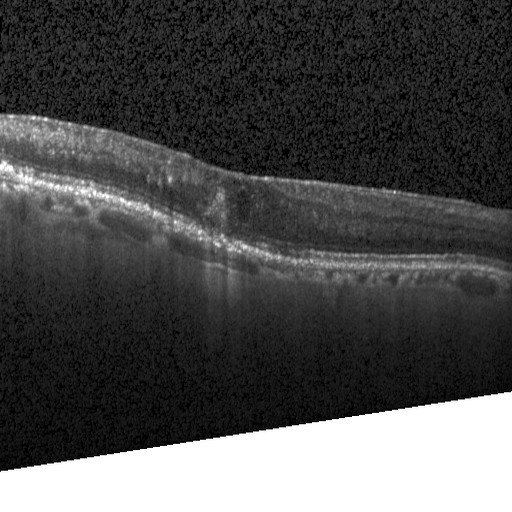 Assessment: DME.